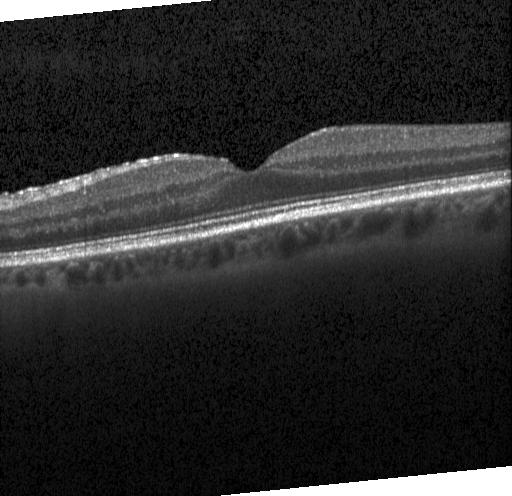
Optical coherence tomography scan. Finding: neither choroidal neovascularization, diabetic macular edema, nor drusen.